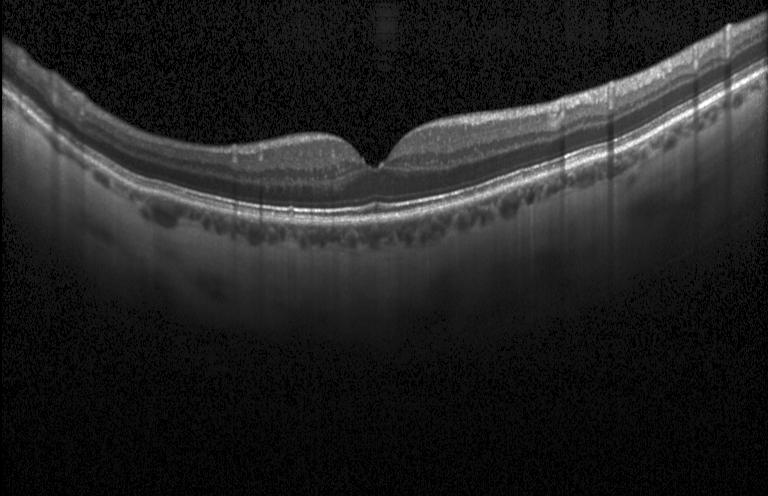
OCT line scan — No CNV, DME, or drusen.